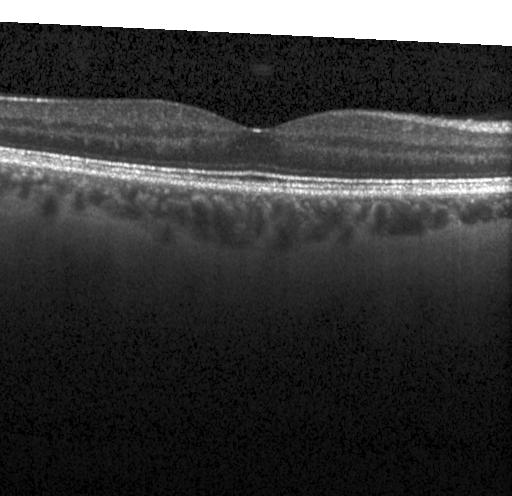
Finding: no evidence of choroidal neovascularization, diabetic macular edema, or drusen.